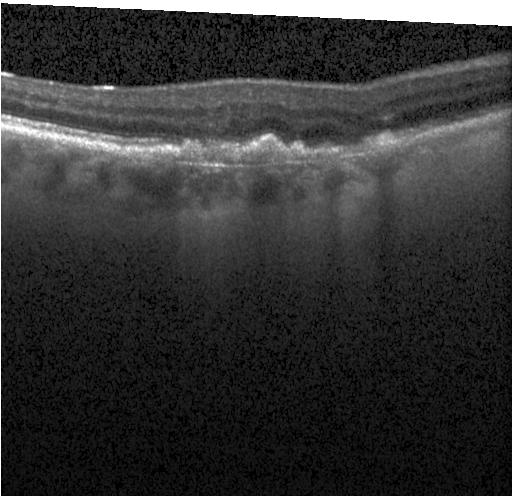 Finding: a choroidal neovascular membrane.